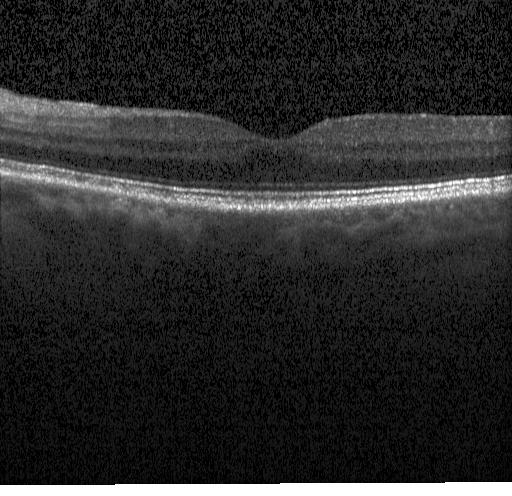 OCT finding: no CNV, DME, or drusen.